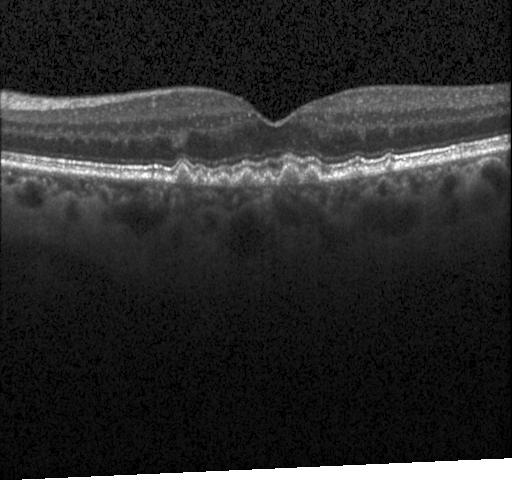
OCT B-scan. Instrument: Heidelberg Spectralis. Horizontal scan through the fovea. SD-OCT.
Dx: sub-RPE drusenoid deposits.